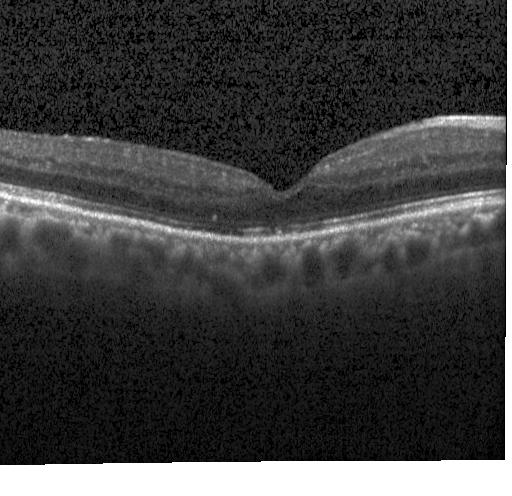
Acquired on a Heidelberg Spectralis, fovea-centered, spectral-domain OCT, retinal OCT B-scan. No evidence of choroidal neovascularization, diabetic macular edema, or drusen.